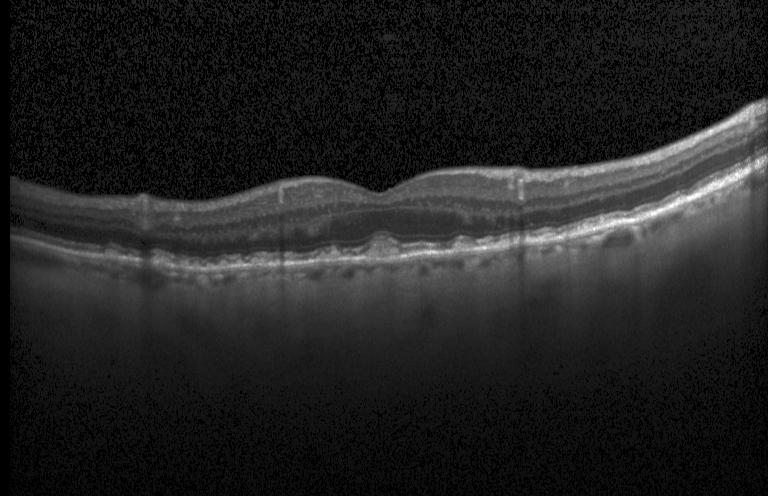 Through the macula, spectral-domain optical coherence tomography, retinal OCT cross-section
Diagnosis: drusen.